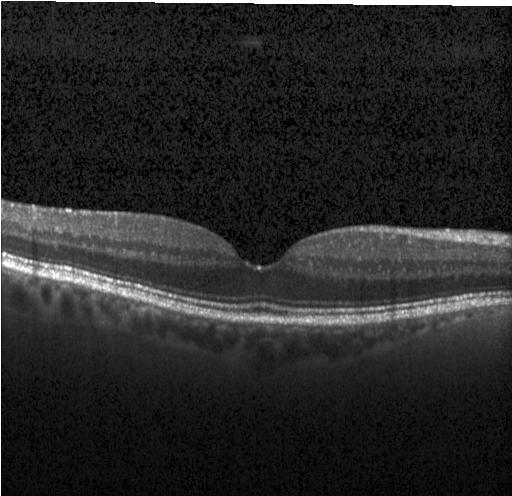 Optical coherence tomography B-scan. Macular OCT: no choroidal neovascularization, diabetic macular edema, or drusen.